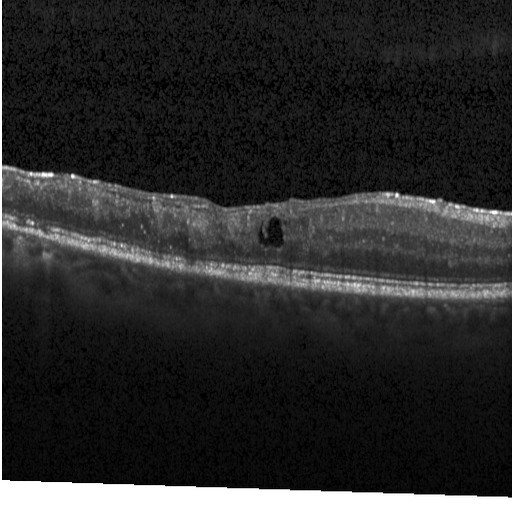

Retinal OCT cross-section — Diagnosis: diabetic macular edema.